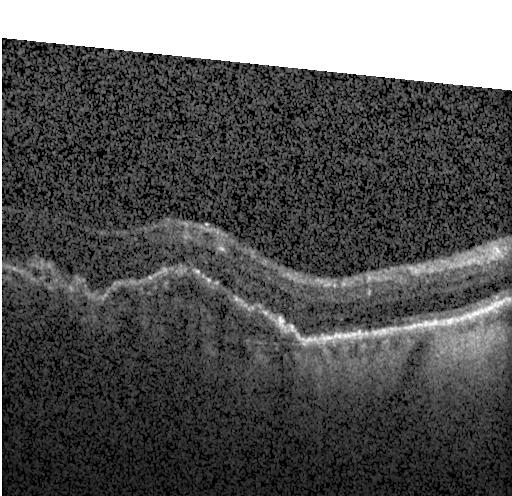 The scan shows choroidal neovascularization (CNV).